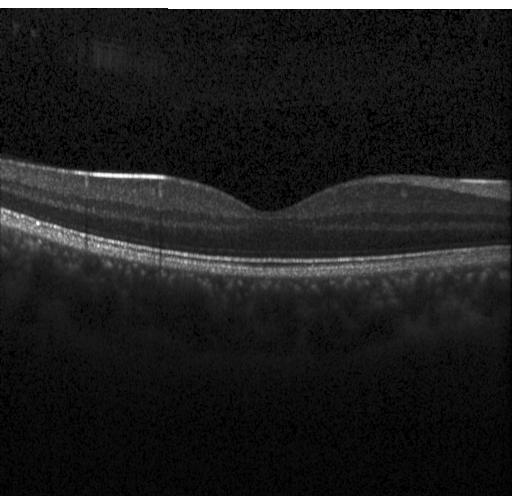 Retinal OCT B-scan — OCT finding: neither choroidal neovascularization, diabetic macular edema, nor drusen.